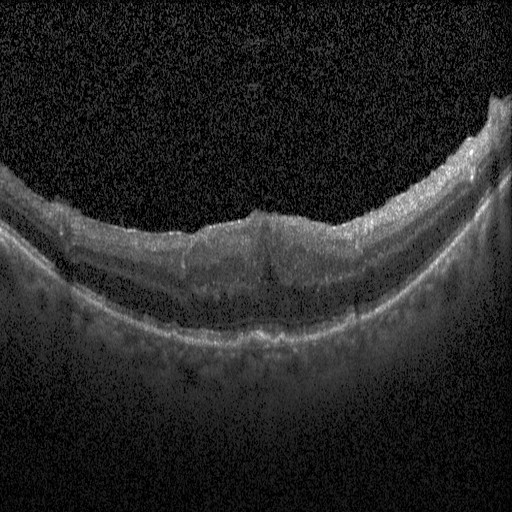

The scan shows diabetic macular edema.